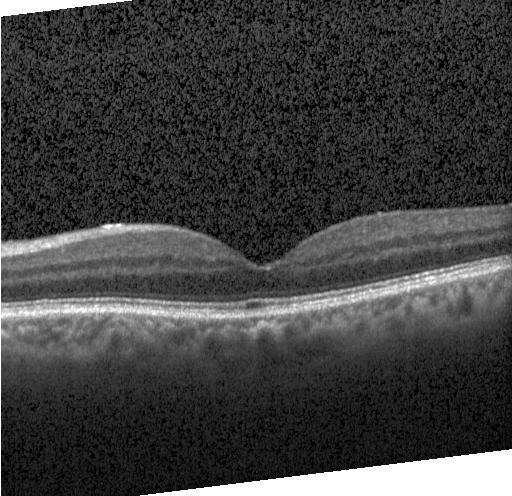 Optical coherence tomography B-scan. Finding: no evidence of choroidal neovascularization, diabetic macular edema, or drusen.